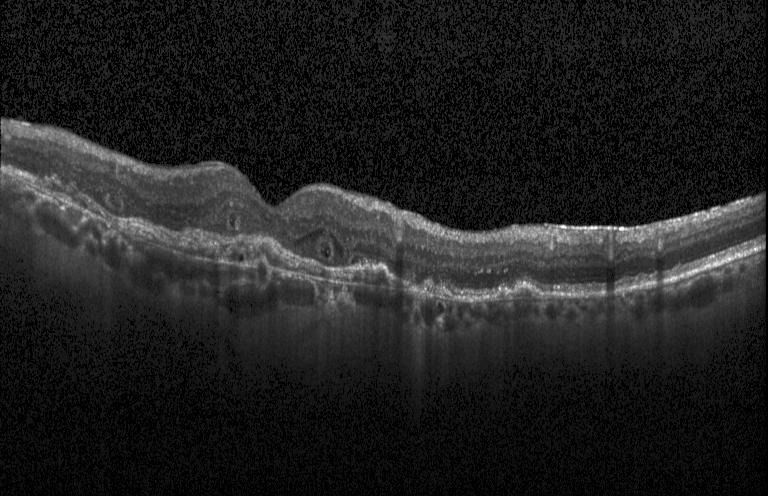 Spectral-domain OCT; Heidelberg Spectralis OCT system; optical coherence tomography scan.
Impression: choroidal neovascularization.